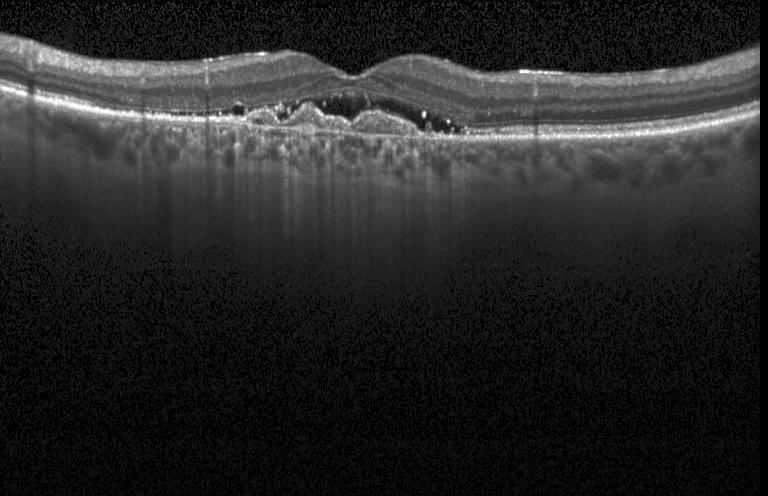 Macular OCT demonstrating a choroidal neovascular membrane.